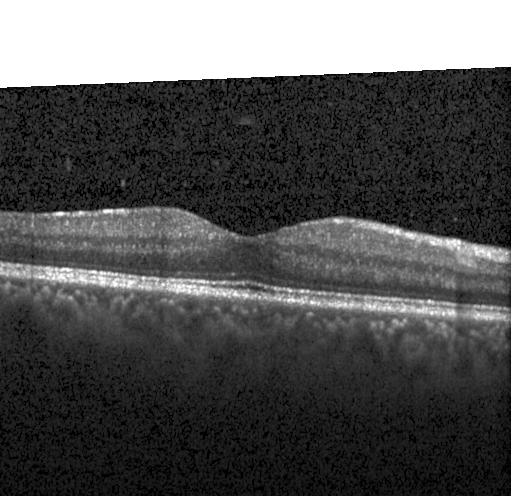

Instrument: Heidelberg Spectralis · optical coherence tomography scan
Finding: no choroidal neovascularization, no diabetic macular edema, and no drusen.